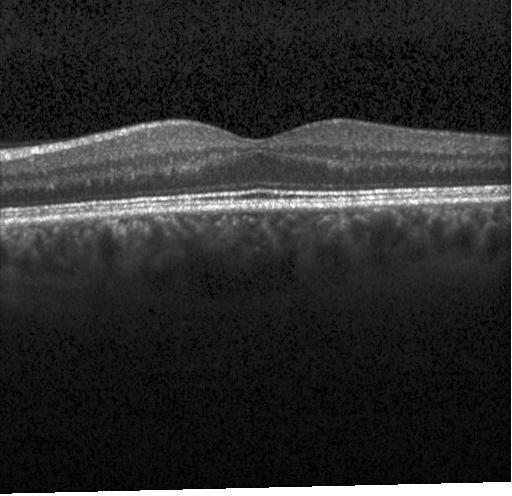 Horizontal scan through the fovea, OCT B-scan, spectral-domain optical coherence tomography.
Impression: no evidence of choroidal neovascularization, diabetic macular edema, or drusen.